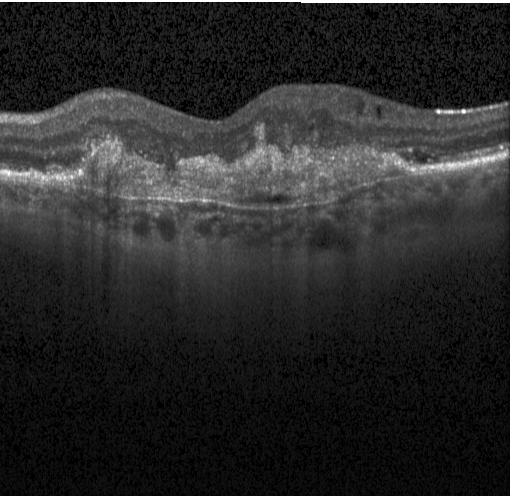
OCT B-scan showing a choroidal neovascular membrane.